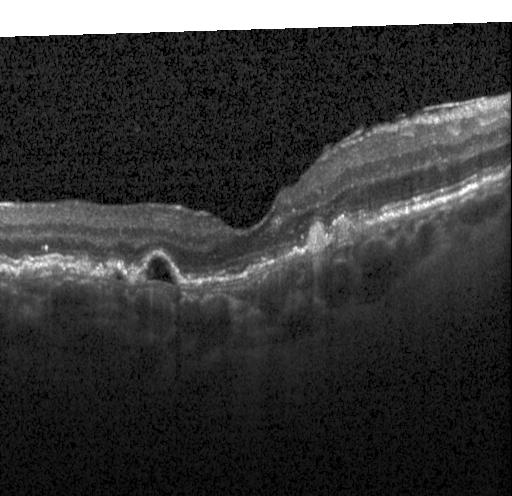
Finding: CNV.